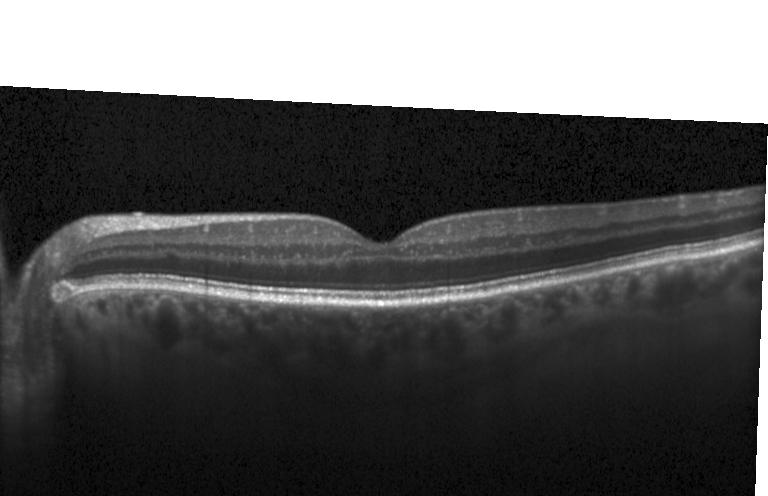 Retinal OCT B-scan, horizontal scan through the fovea, instrument: Heidelberg Spectralis
Macular OCT: no choroidal neovascularization, diabetic macular edema, or drusen.